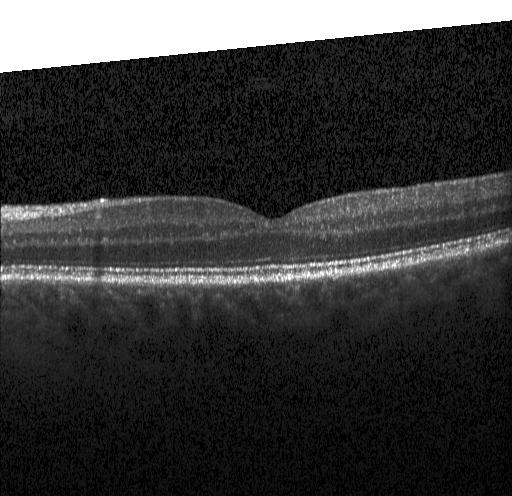 Diagnosis: no evidence of CNV, DME, or drusen.